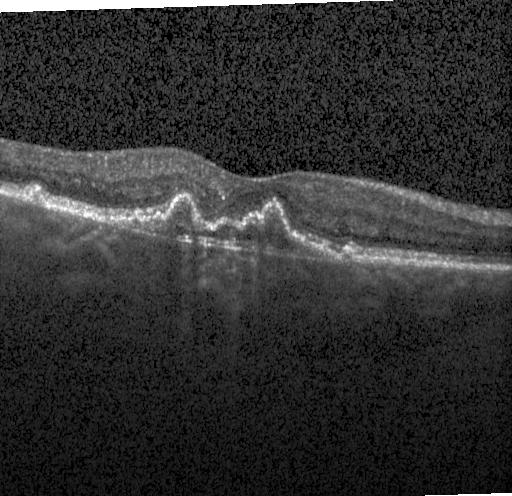

Diagnosis: CNV.